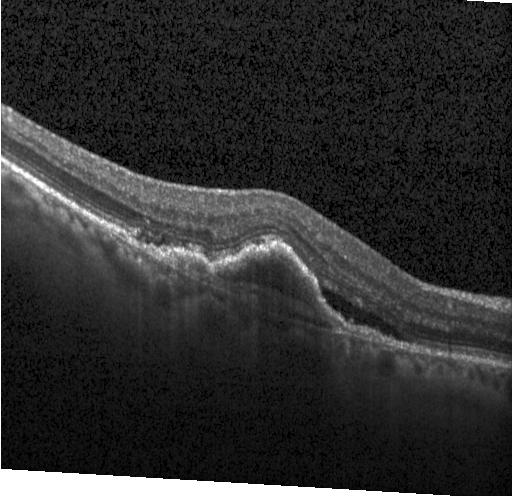
OCT B-scan — Assessment: a choroidal neovascular membrane.